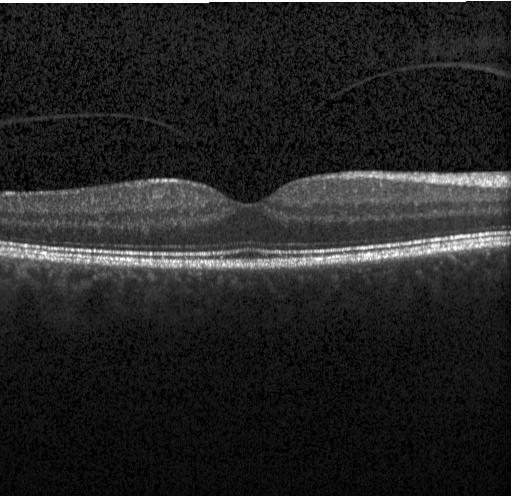

Impression: neither CNV, DME, nor drusen.